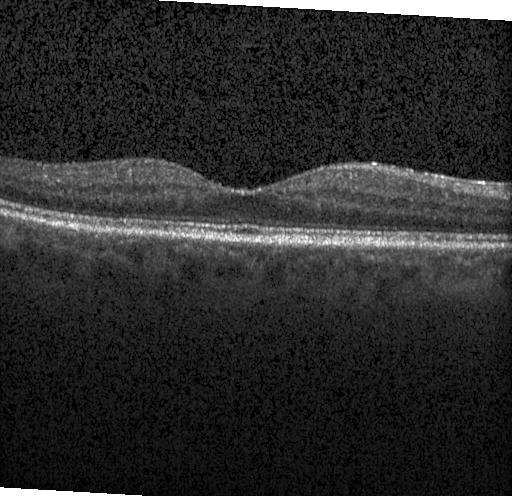
Centered on the fovea, instrument: Heidelberg Spectralis, OCT B-scan
Impression: no evidence of choroidal neovascularization, diabetic macular edema, or drusen.